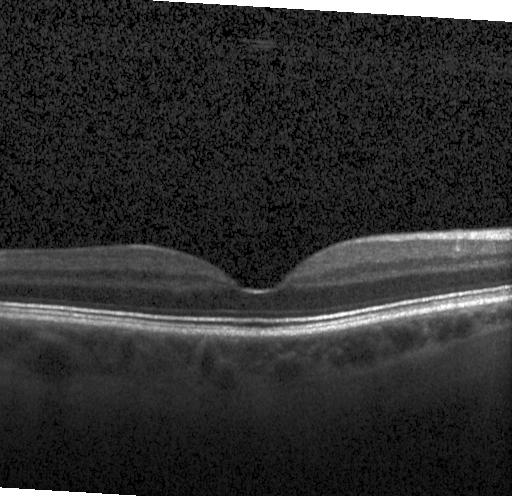

Impression: no CNV, DME, or drusen.